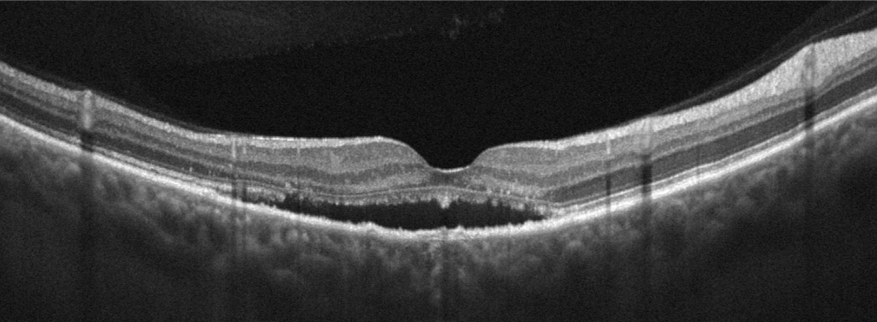
OCT line scan · instrument: Optovue Avanti RTVue XR · fovea-centered. Dx: AMD.